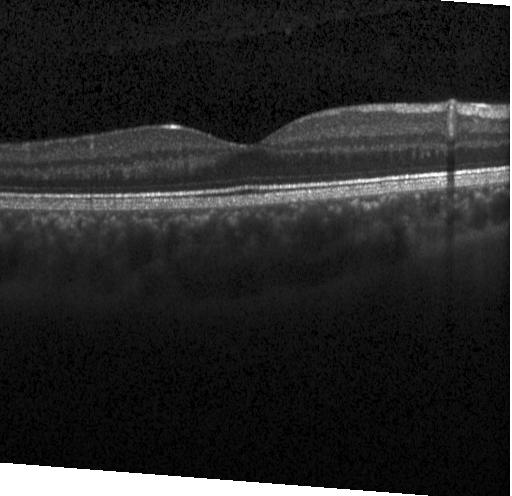

OCT B-scan showing neither CNV, DME, nor drusen.